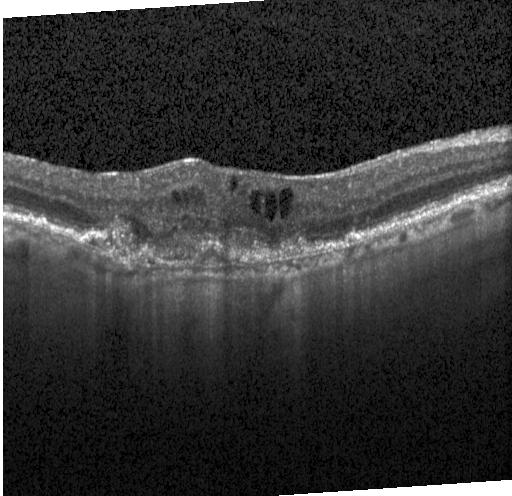 Through the macula. Acquired on a Heidelberg Spectralis. Optical coherence tomography scan — Assessment: choroidal neovascularization.